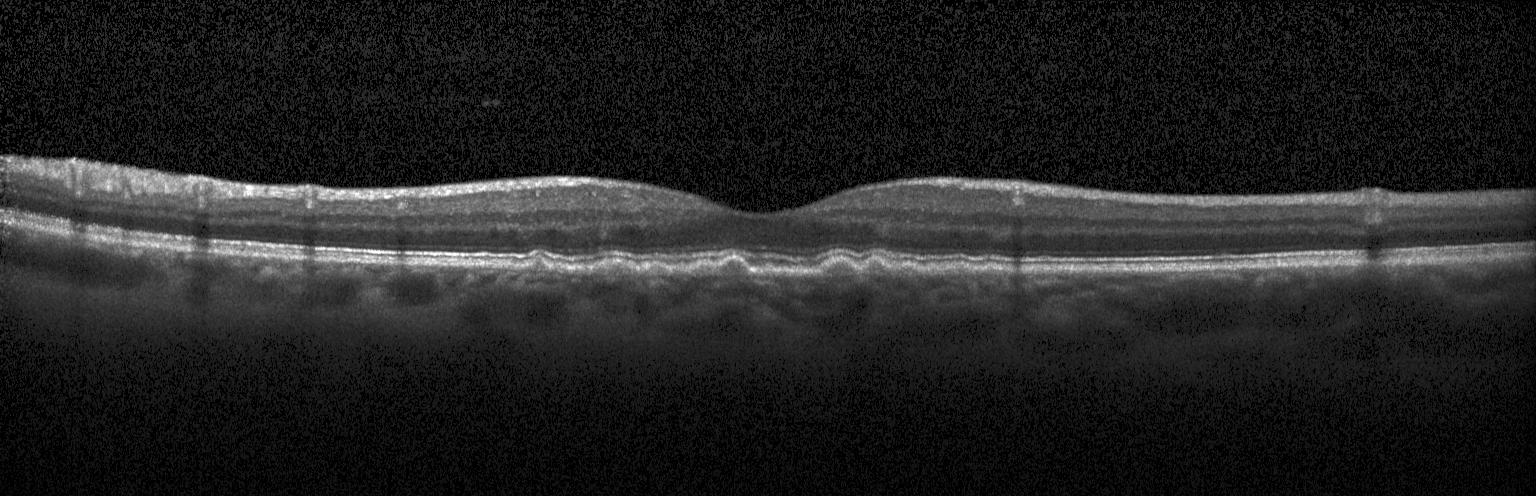

Dx: drusen.